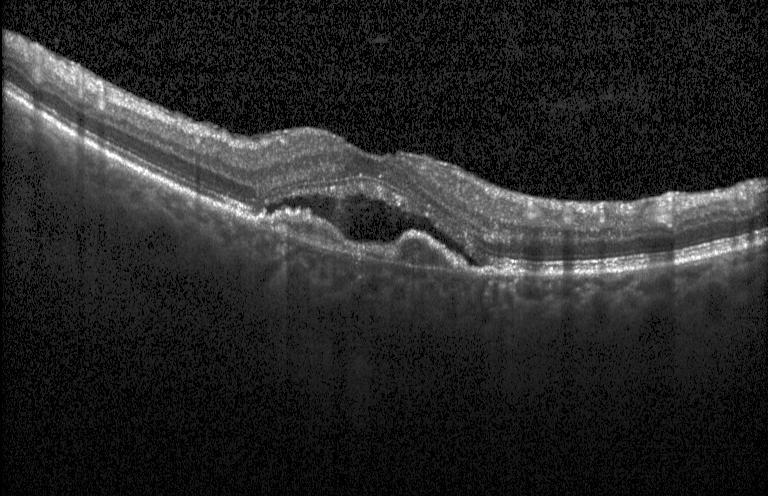

Instrument: Heidelberg Spectralis, retinal OCT cross-section, fovea-centered — Macular OCT: a choroidal neovascular membrane.